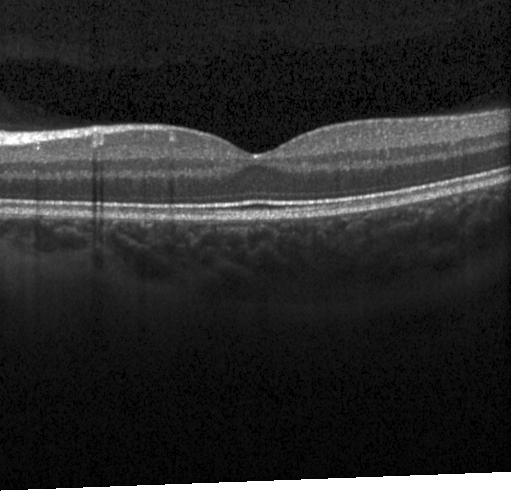
No choroidal neovascularization, diabetic macular edema, or drusen.